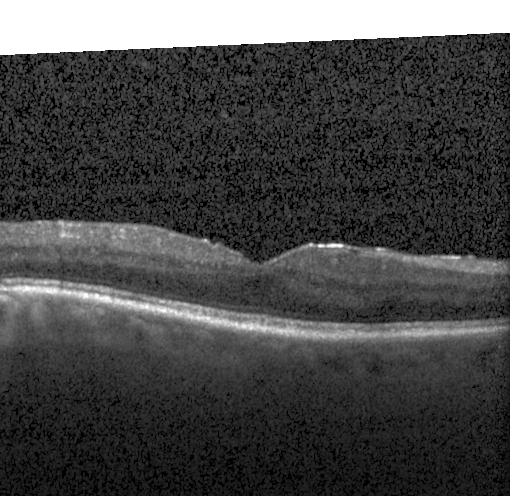 Horizontal scan through the fovea. Spectral-domain optical coherence tomography. Optical coherence tomography B-scan — OCT finding: no evidence of CNV, DME, or drusen.